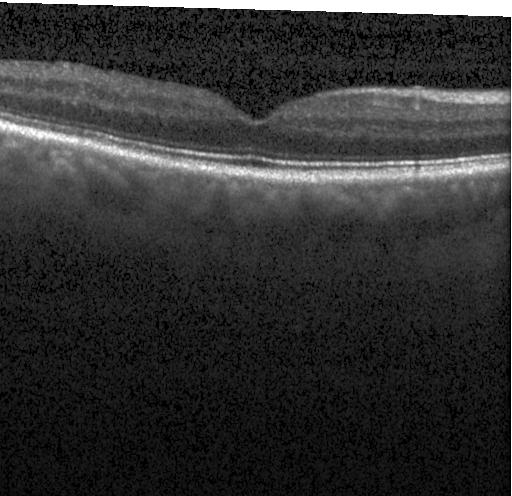

Retinal OCT B-scan, centered on the fovea — The scan shows no evidence of choroidal neovascularization, diabetic macular edema, or drusen.